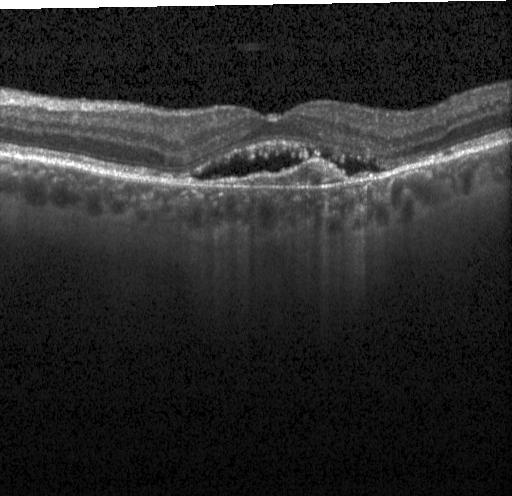
Finding: CNV.